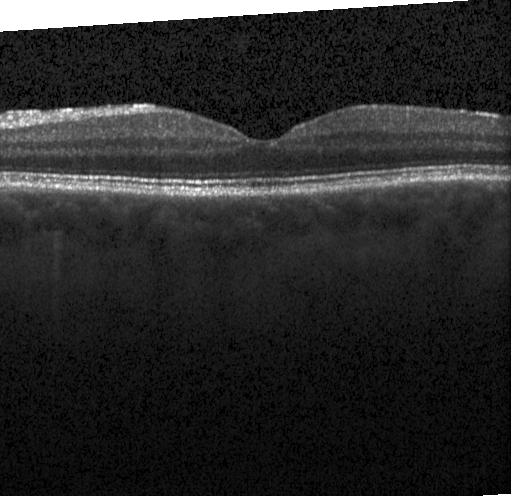
OCT B-scan.
OCT finding: no choroidal neovascularization, no diabetic macular edema, and no drusen.